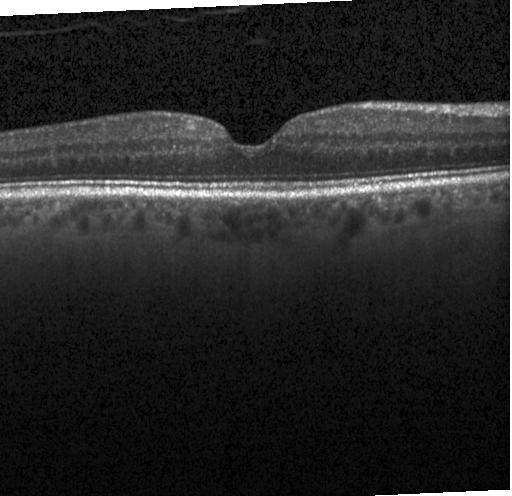

Macular OCT demonstrating no choroidal neovascularization, no diabetic macular edema, and no drusen.